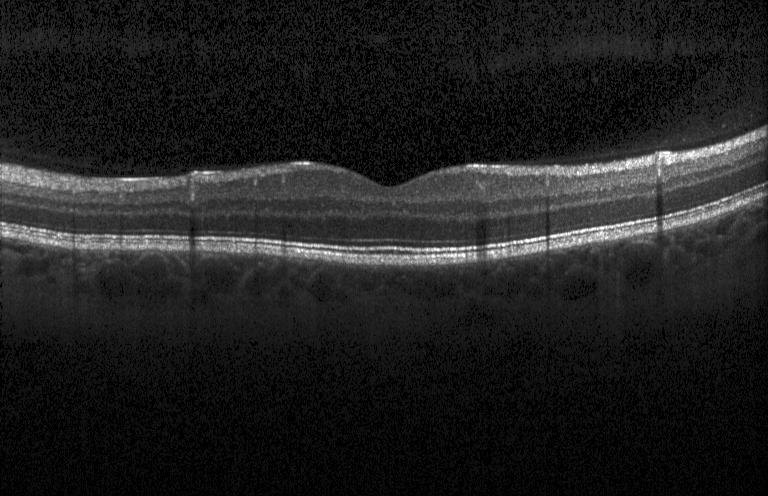 Optical coherence tomography B-scan
Dx: neither choroidal neovascularization, diabetic macular edema, nor drusen.